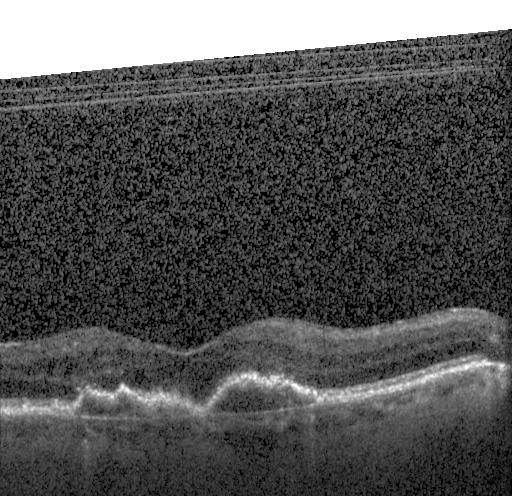
Retinal OCT cross-section
Diagnosis: CNV.